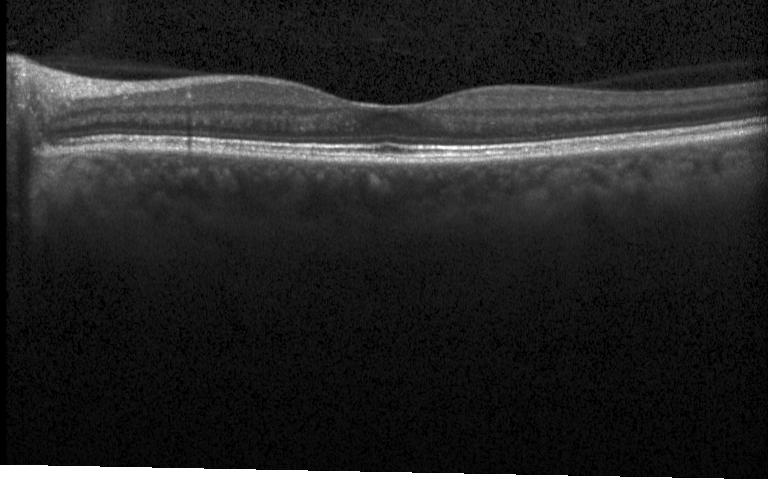 Assessment: neither choroidal neovascularization, diabetic macular edema, nor drusen.